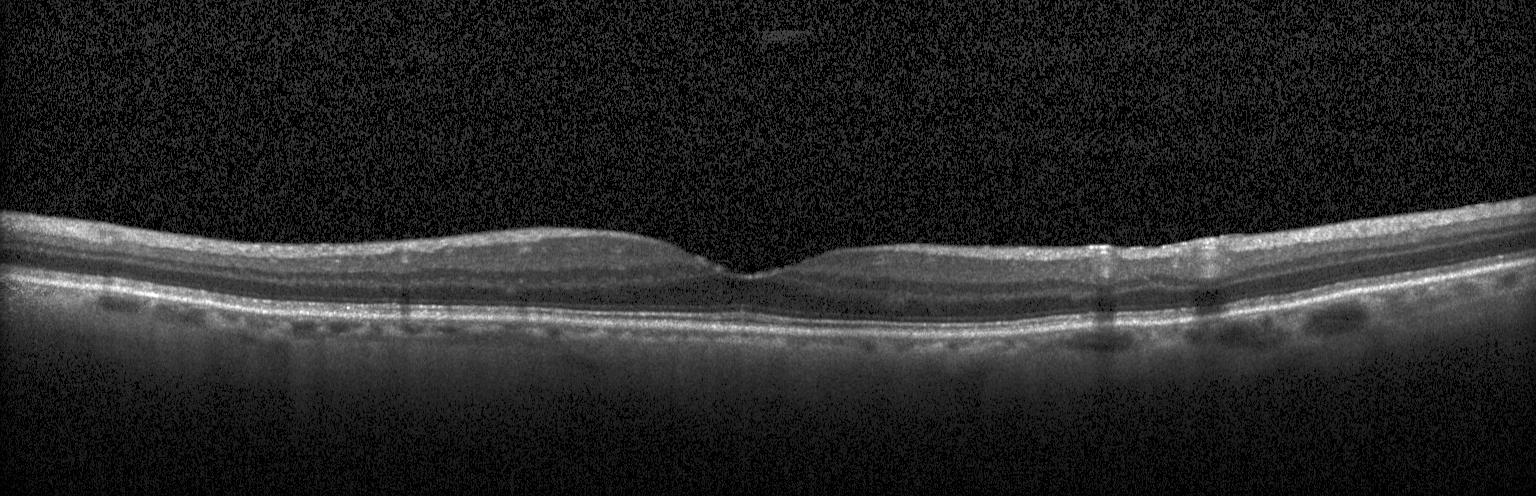
Retinal OCT cross-section.
Assessment: no choroidal neovascularization, diabetic macular edema, or drusen.